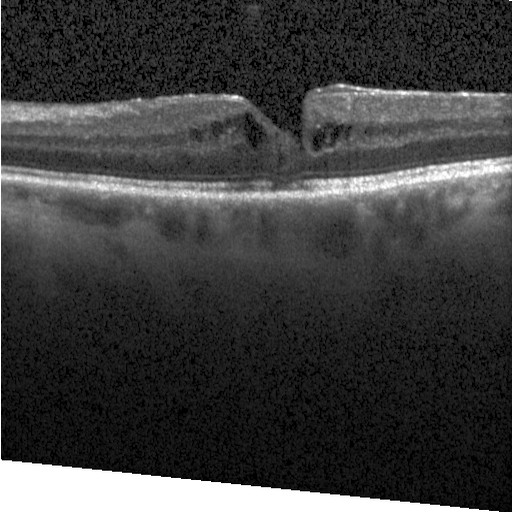
OCT B-scan.
The scan shows DME.